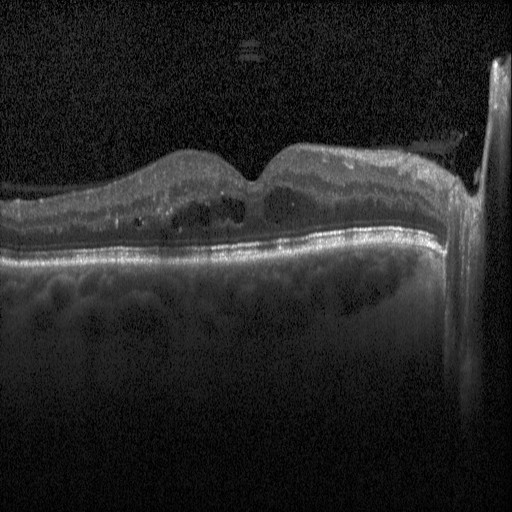 Macular OCT: diabetic macular edema (DME).